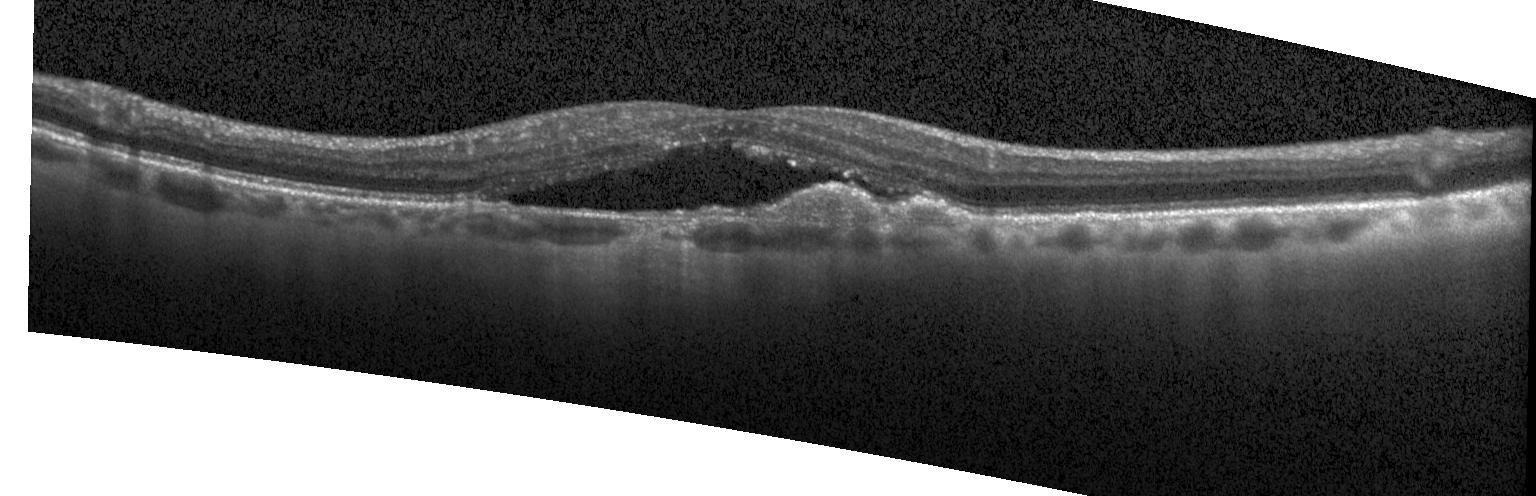

Heidelberg Spectralis OCT system · OCT B-scan
Diagnosis: CNV.